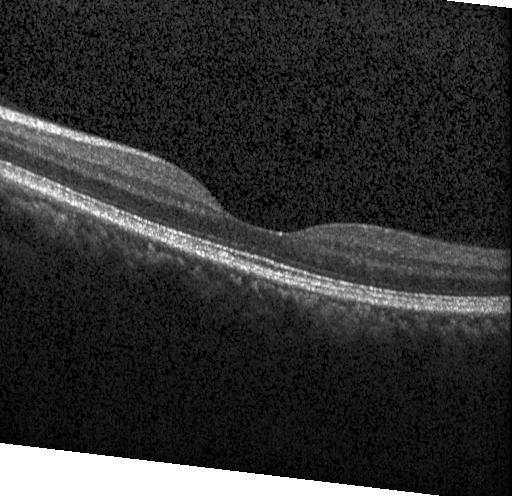 Dx: no choroidal neovascularization, no diabetic macular edema, and no drusen.